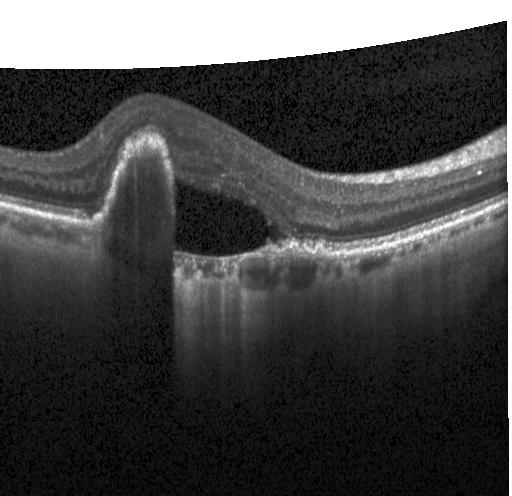
Assessment: a choroidal neovascular membrane.